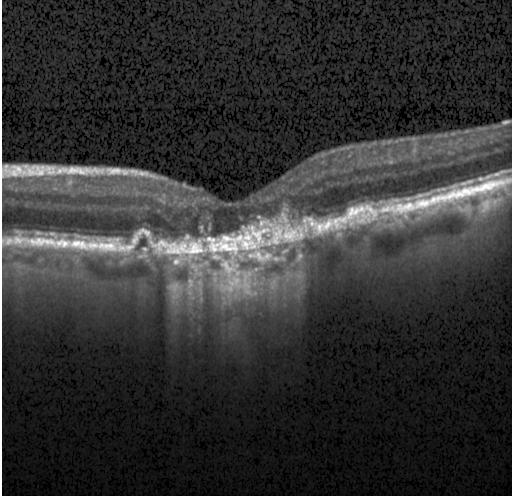 Optical coherence tomography scan — This B-scan demonstrates a choroidal neovascular membrane.